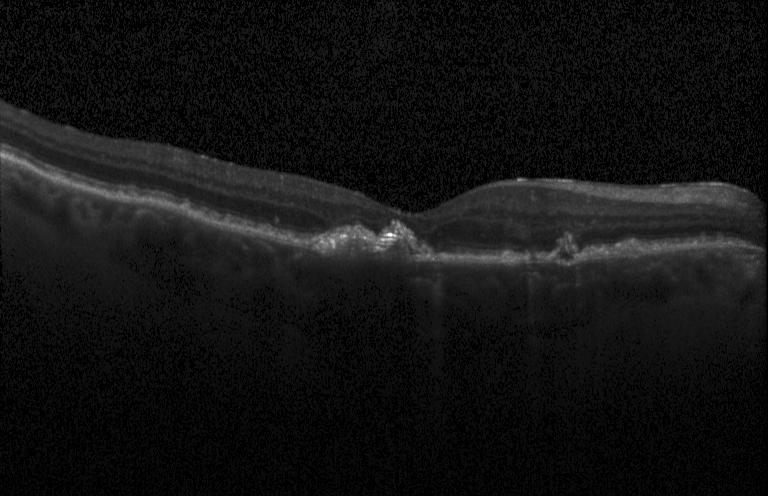

Dx: CNV.